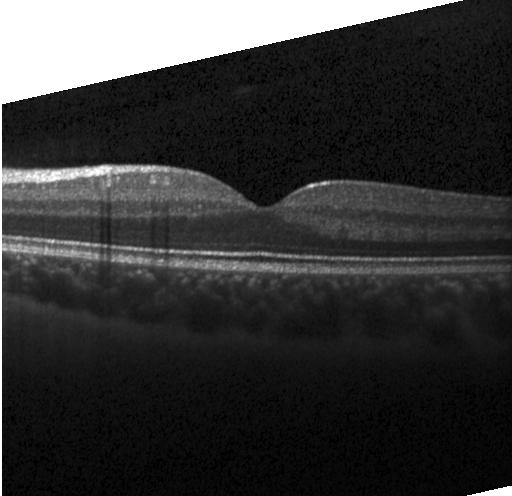
Impression: neither choroidal neovascularization, diabetic macular edema, nor drusen.